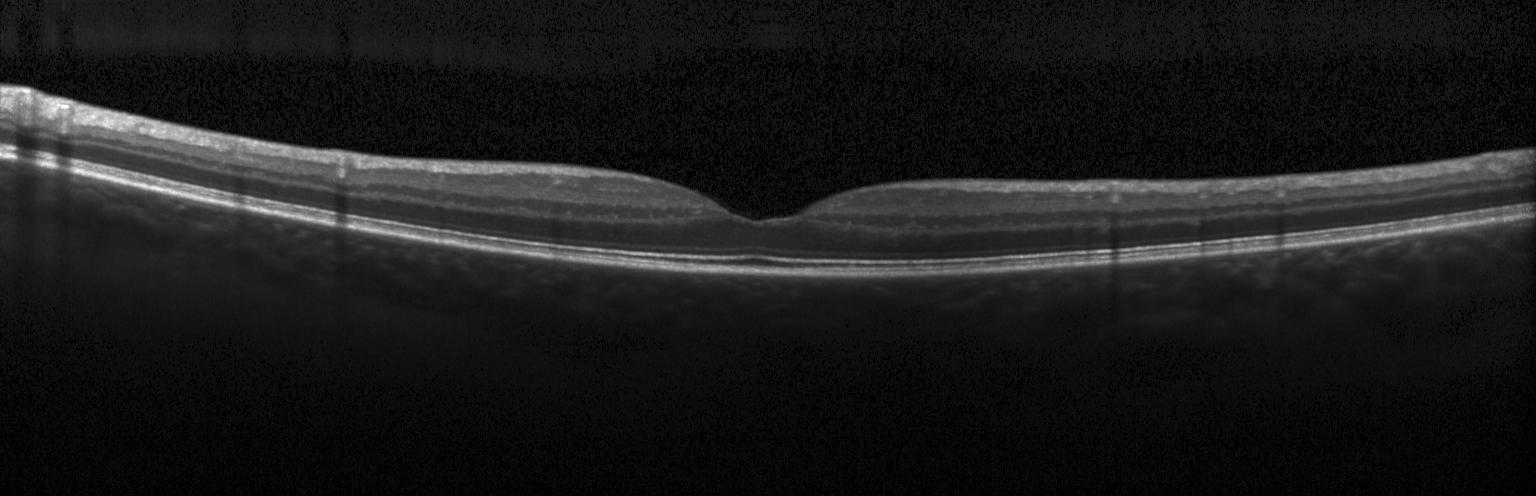 OCT finding: no evidence of choroidal neovascularization, diabetic macular edema, or drusen.